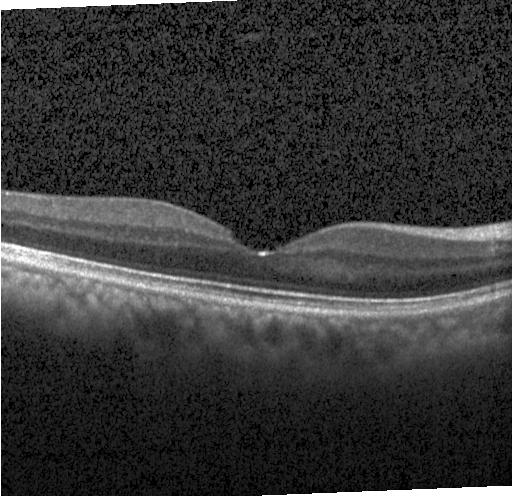

Dx: no choroidal neovascularization, diabetic macular edema, or drusen.